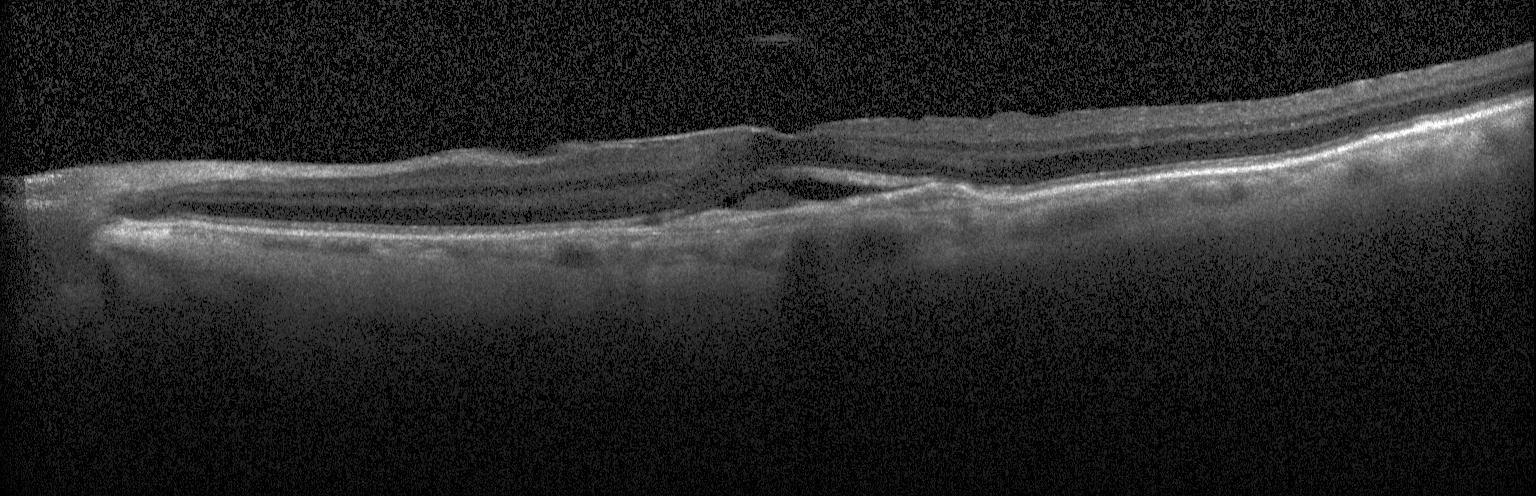

OCT B-scan, fovea-centered.
Dx: a choroidal neovascular membrane.